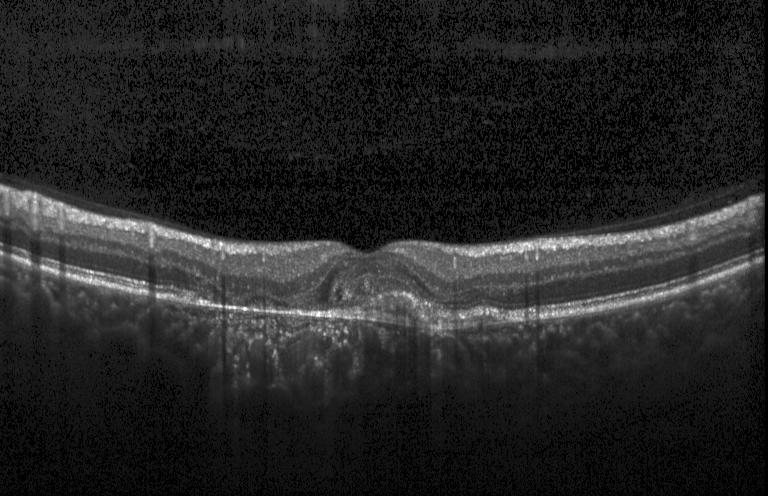 Spectral-domain OCT, optical coherence tomography scan. Assessment: choroidal neovascularization (CNV).